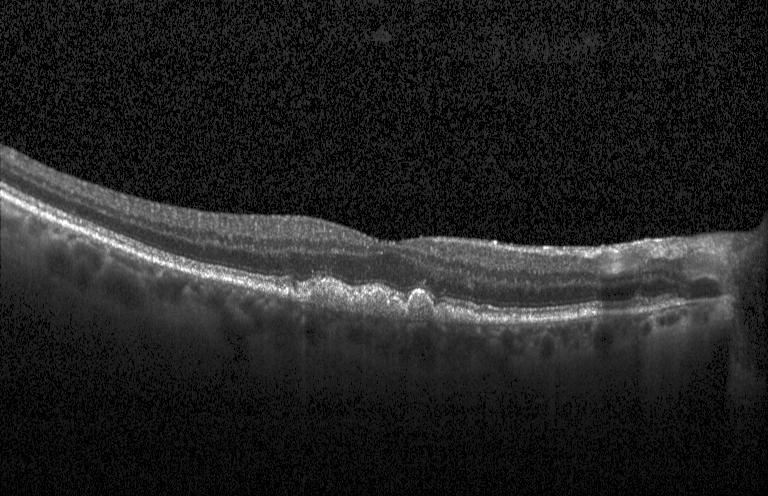 Through the macula, OCT B-scan, Heidelberg Spectralis, spectral-domain OCT
Finding: drusen.